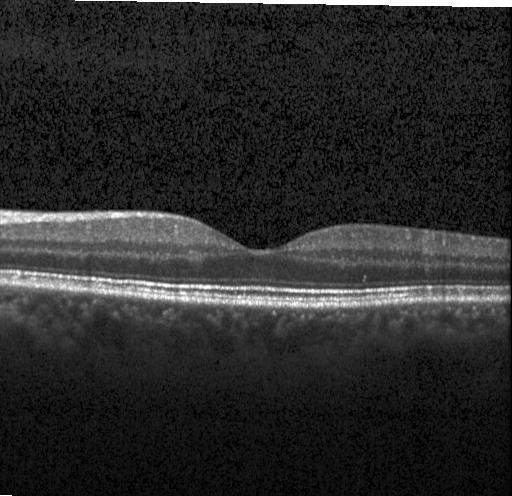 Heidelberg Spectralis; fovea-centered; retinal OCT cross-section.
The scan shows no evidence of choroidal neovascularization, diabetic macular edema, or drusen.